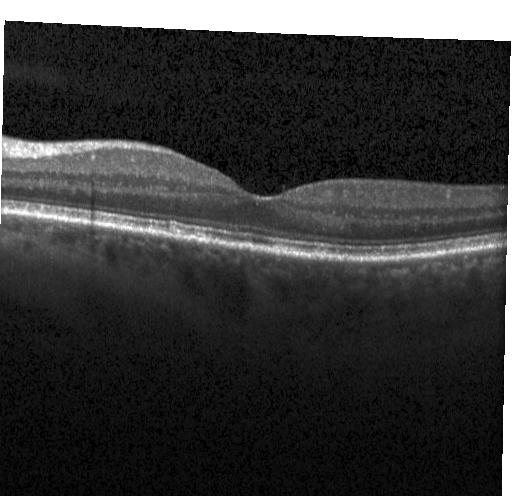 No choroidal neovascularization, no diabetic macular edema, and no drusen.